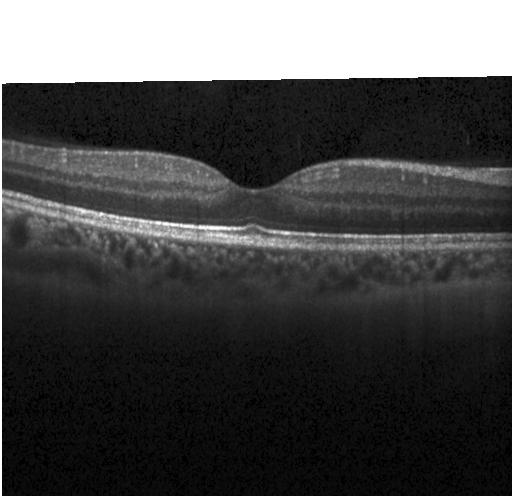
OCT B-scan, spectral-domain optical coherence tomography.
Diagnosis: neither choroidal neovascularization, diabetic macular edema, nor drusen.